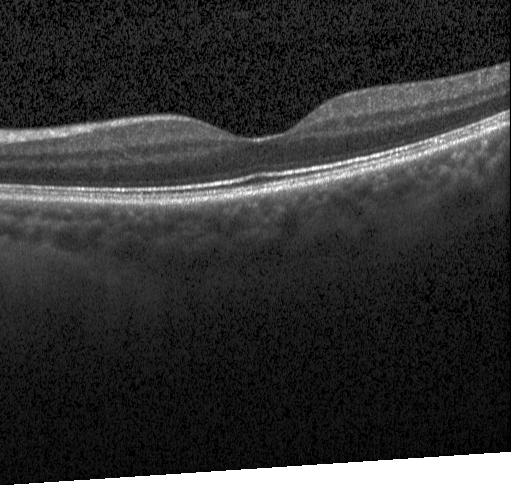

Macular scan, Heidelberg Spectralis, OCT line scan
This B-scan demonstrates neither choroidal neovascularization, diabetic macular edema, nor drusen.